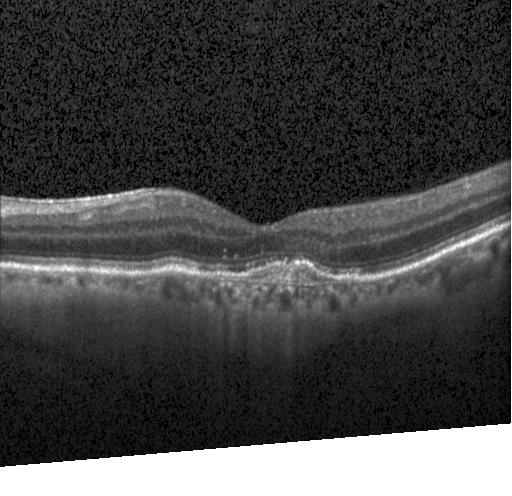
Optical coherence tomography B-scan; horizontal scan through the fovea; Heidelberg Spectralis OCT system; SD-OCT
Dx: a choroidal neovascular membrane.